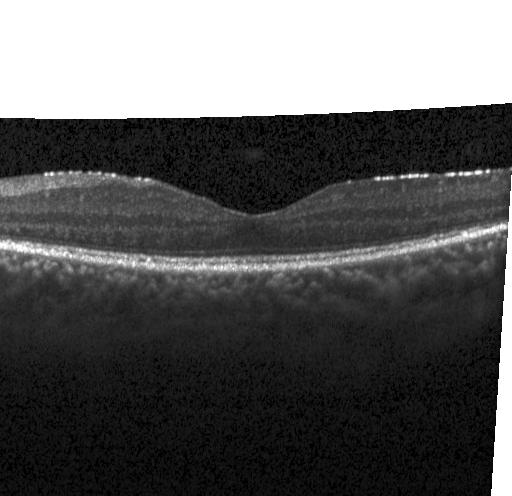
Optical coherence tomography scan · acquired on a Heidelberg Spectralis.
Finding: no evidence of choroidal neovascularization, diabetic macular edema, or drusen.